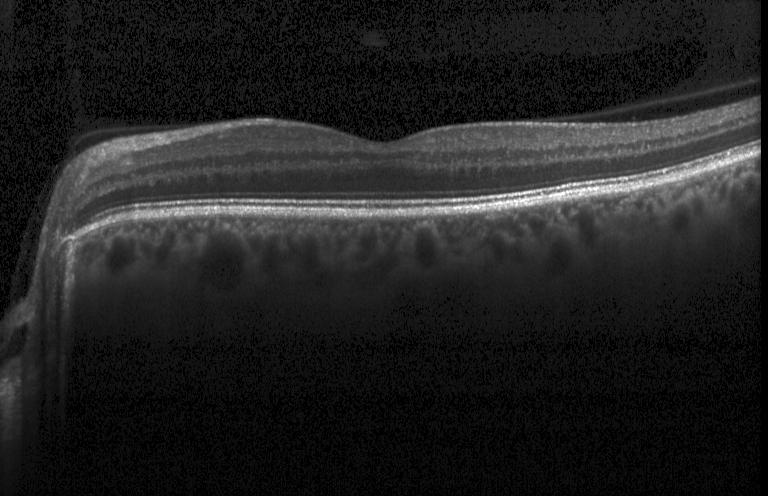 Dx: no evidence of CNV, DME, or drusen.